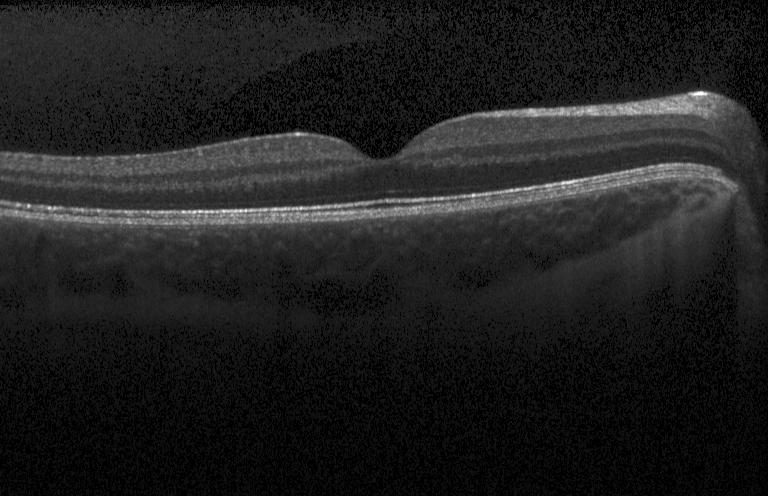
Optical coherence tomography B-scan; spectral-domain optical coherence tomography
No choroidal neovascularization, no diabetic macular edema, and no drusen.